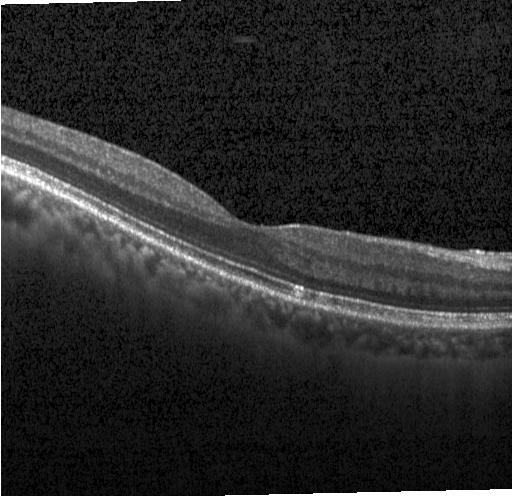
OCT finding: no choroidal neovascularization, diabetic macular edema, or drusen.